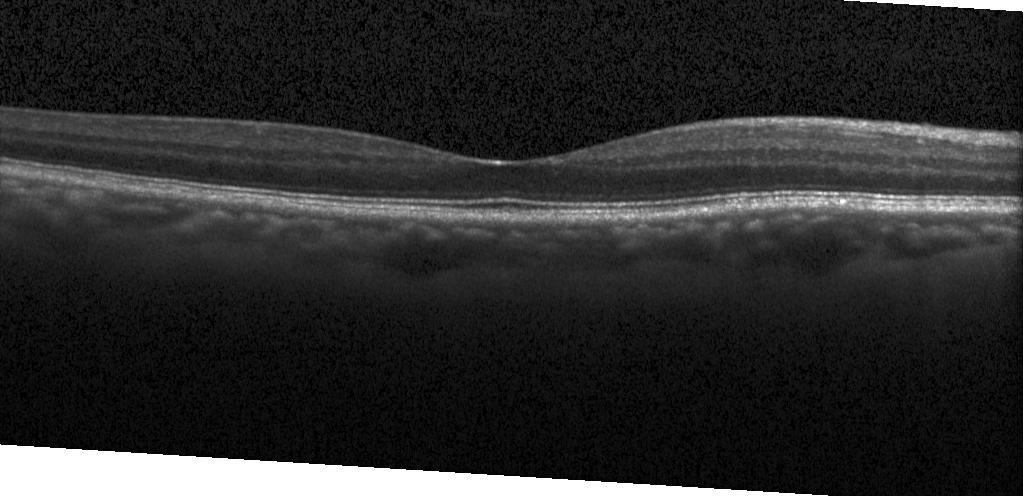

Impression: no choroidal neovascularization, diabetic macular edema, or drusen.